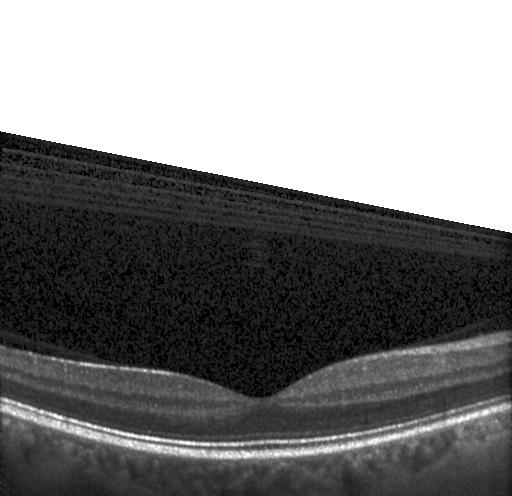 Macular OCT: no choroidal neovascularization, no diabetic macular edema, and no drusen.